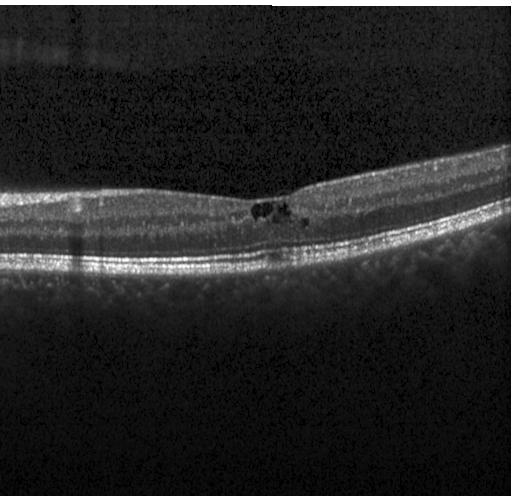
Macular scan, optical coherence tomography scan, spectral-domain OCT, instrument: Heidelberg Spectralis — Diabetic macular edema (DME).